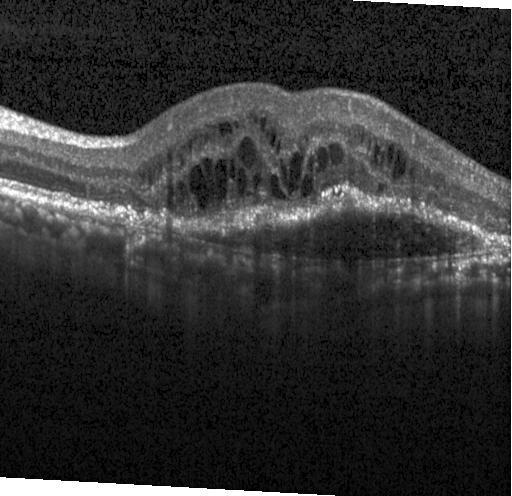 Spectral-domain OCT B-scan: choroidal neovascularization.